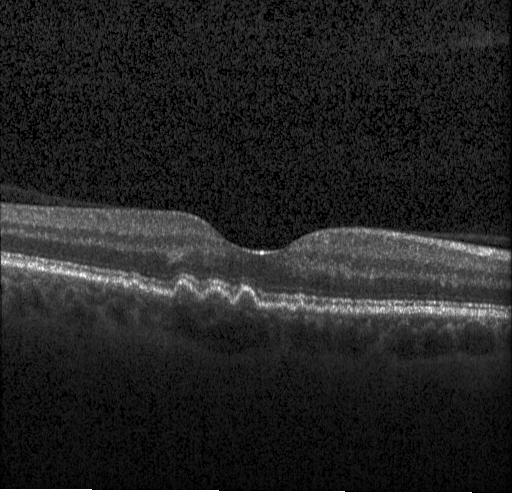 OCT finding: sub-RPE drusenoid deposits.